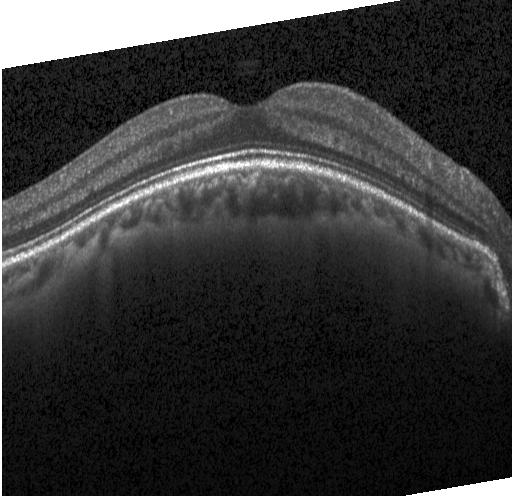

Through the macula, OCT B-scan.
This B-scan demonstrates no CNV, no DME, and no drusen.